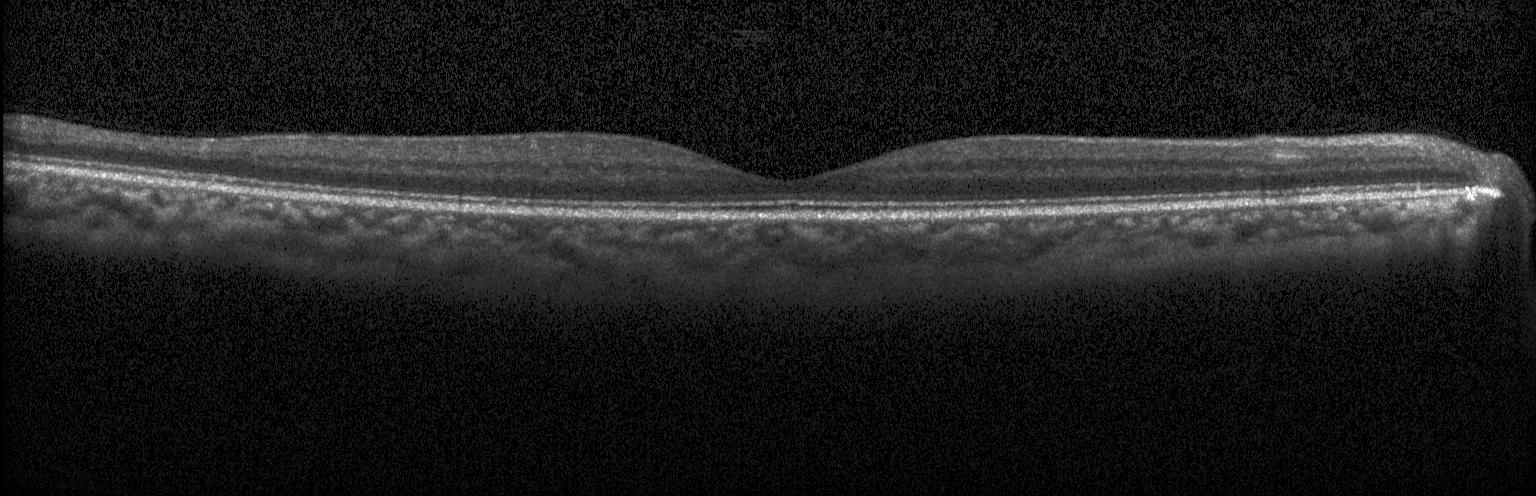
Fovea-centered; SD-OCT; optical coherence tomography scan; instrument: Heidelberg Spectralis. Finding: no choroidal neovascularization, diabetic macular edema, or drusen.